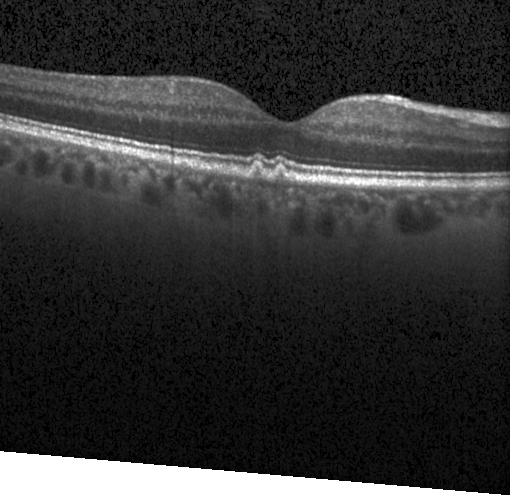 Assessment: sub-RPE drusenoid deposits.